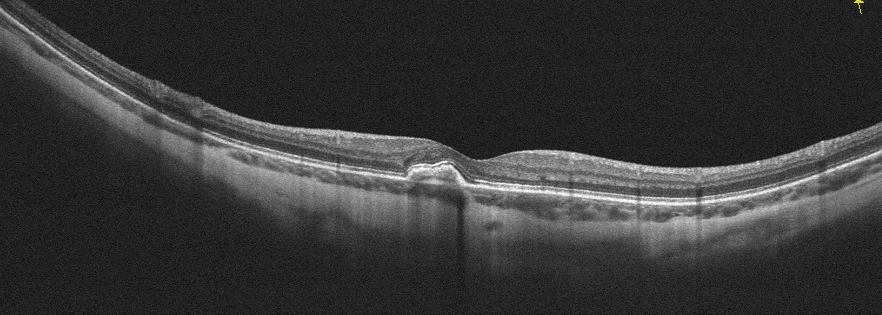

OCT line scan
Finding: AMD.